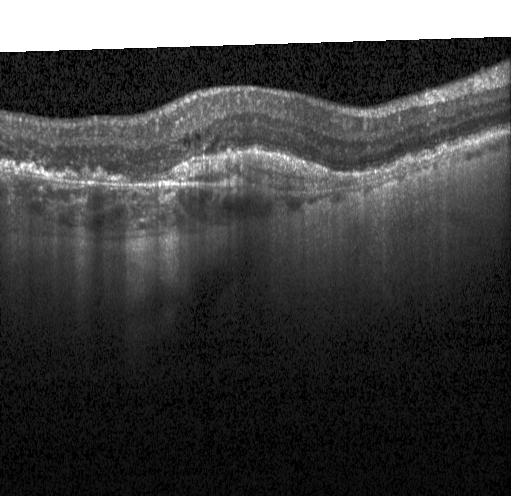
Impression: a choroidal neovascular membrane.